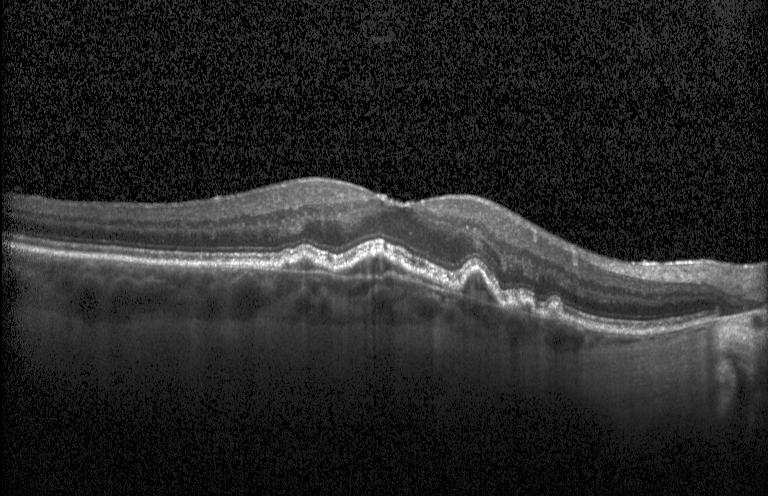 OCT B-scan showing a choroidal neovascular membrane.